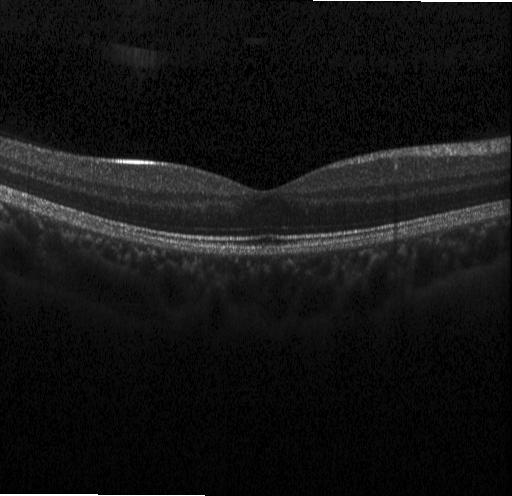
Heidelberg Spectralis. Horizontal scan through the fovea. Optical coherence tomography scan. SD-OCT. Finding: no choroidal neovascularization, diabetic macular edema, or drusen.